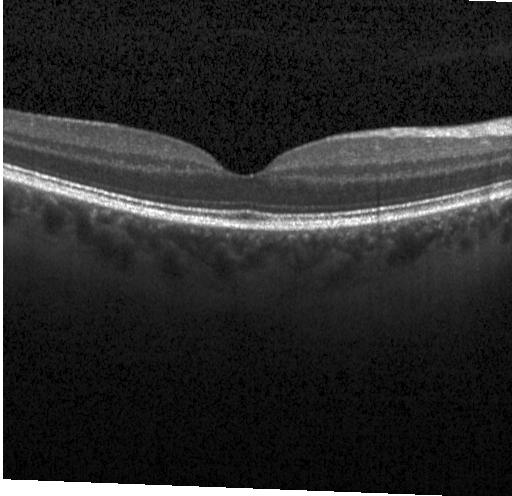

Macular scan · retinal OCT cross-section.
Assessment: neither CNV, DME, nor drusen.